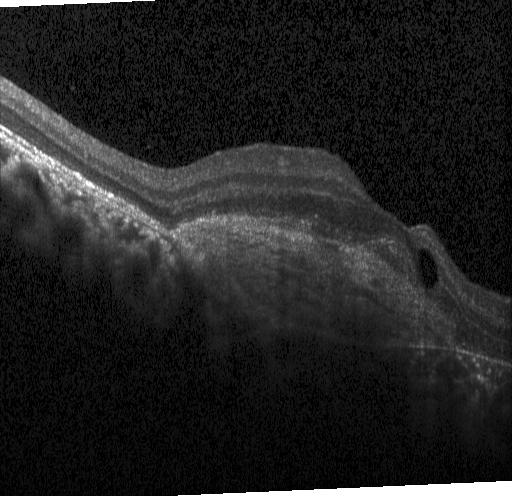
Retinal OCT B-scan. Spectral-domain optical coherence tomography. Instrument: Heidelberg Spectralis — This B-scan demonstrates a choroidal neovascular membrane.